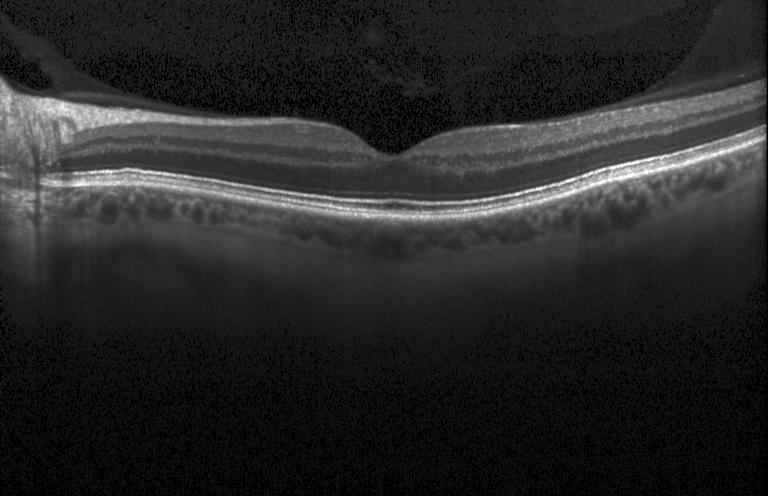

Retinal OCT cross-section. OCT finding: no choroidal neovascularization, diabetic macular edema, or drusen.